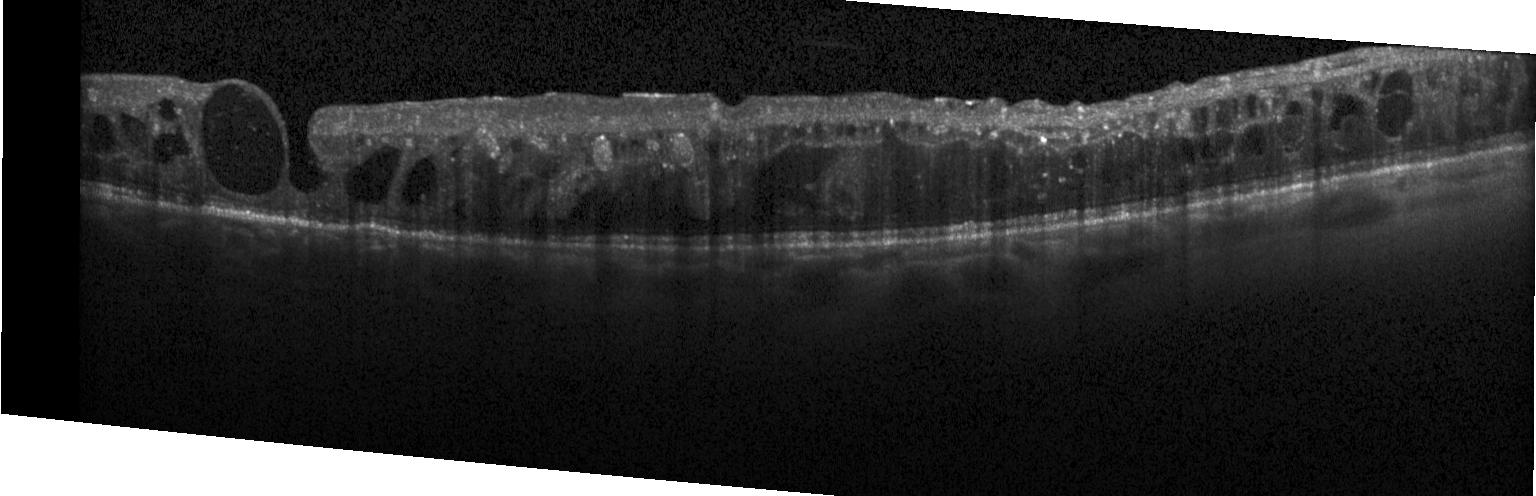
Diagnosis: DME.